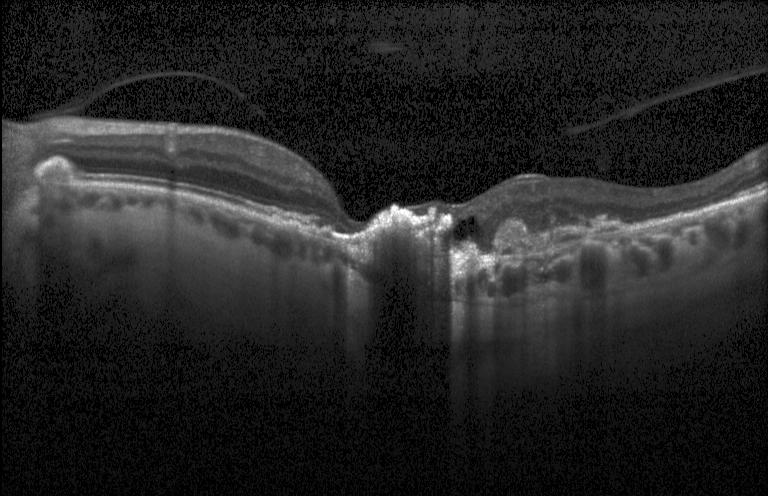 Dx: a choroidal neovascular membrane.